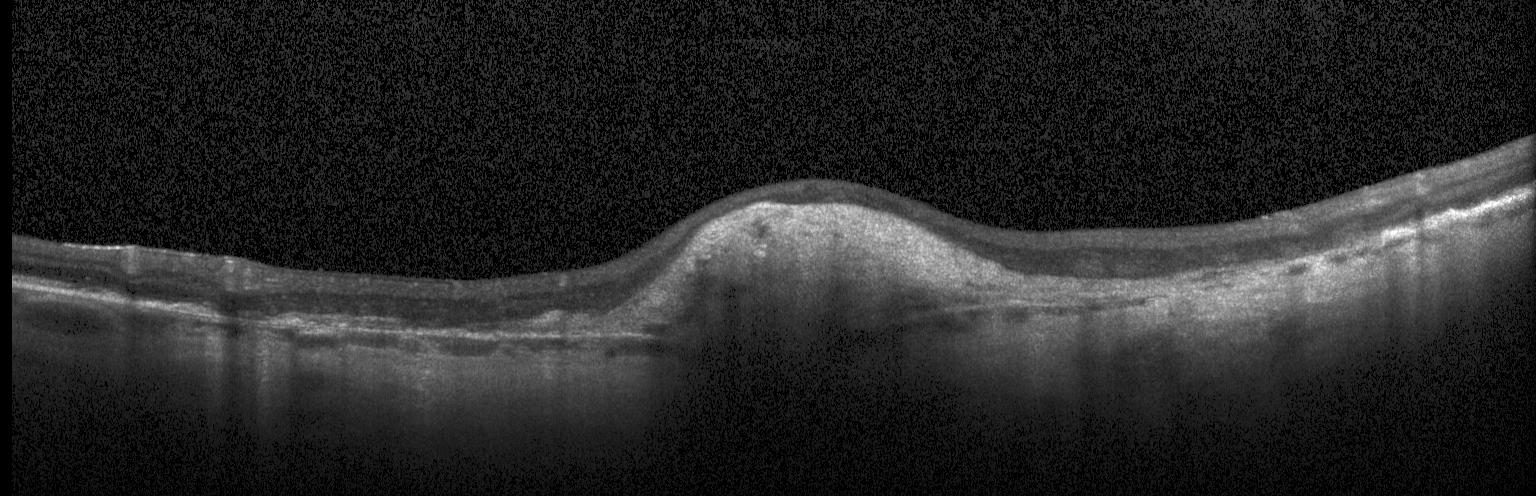

Diagnosis: a choroidal neovascular membrane.